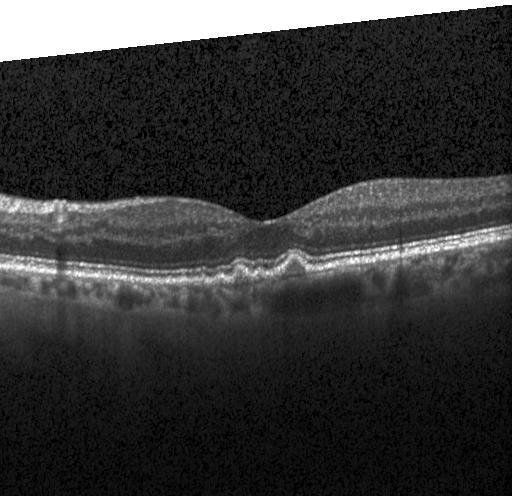
Optical coherence tomography scan · fovea-centered · Heidelberg Spectralis. OCT finding: multiple drusen.